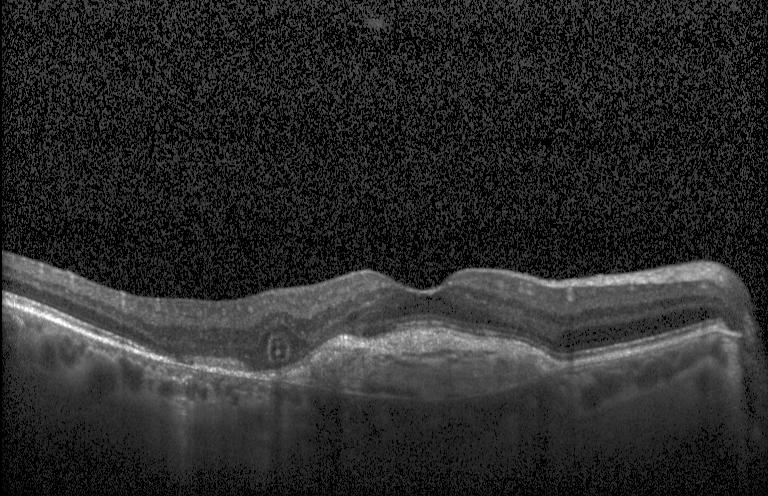

Macular scan, optical coherence tomography B-scan, spectral-domain OCT — Choroidal neovascularization (CNV).